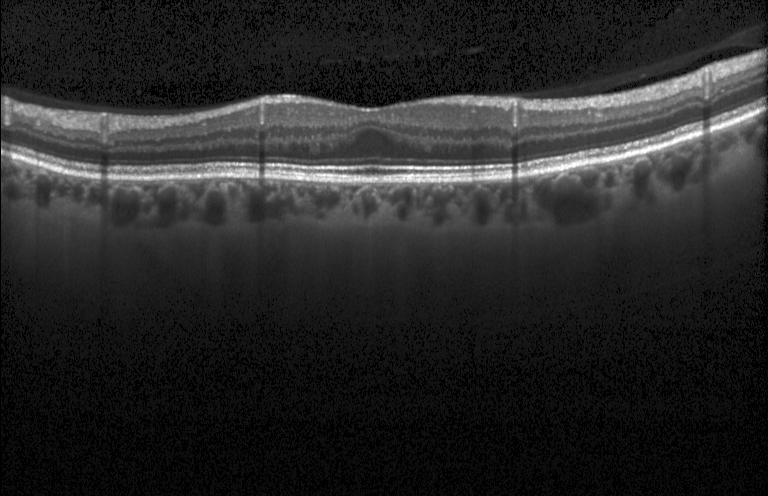 Assessment: no choroidal neovascularization, no diabetic macular edema, and no drusen.